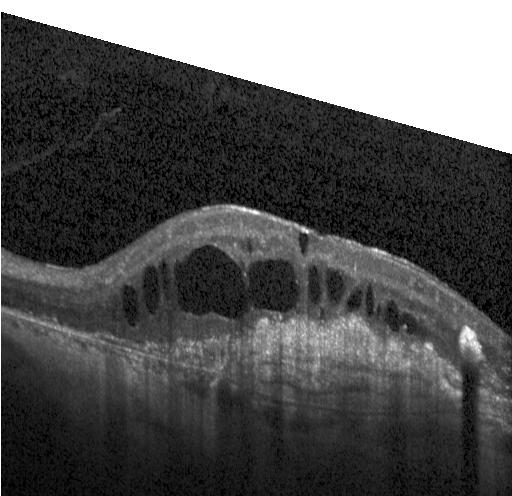 Retinal OCT B-scan; SD-OCT — Impression: a choroidal neovascular membrane.